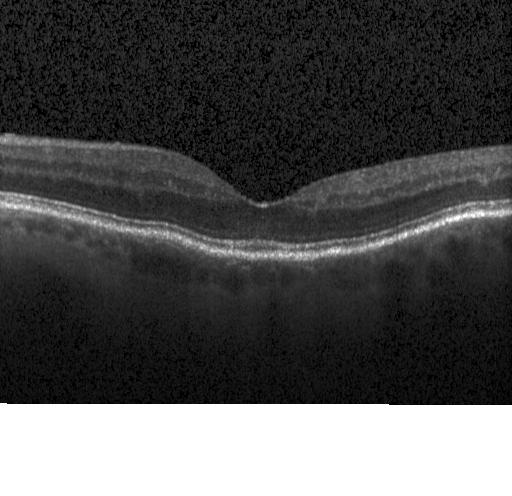

Spectral-domain OCT B-scan: no evidence of choroidal neovascularization, diabetic macular edema, or drusen.